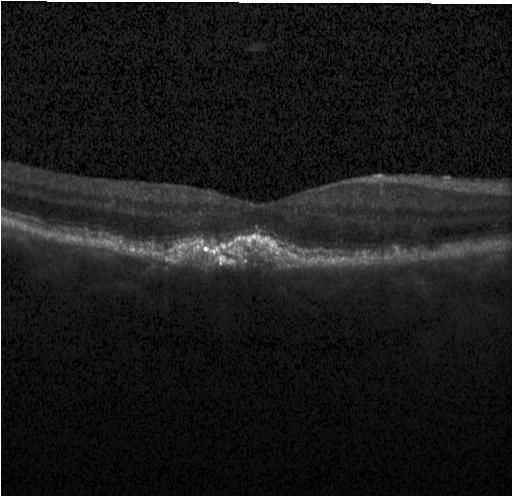 Heidelberg Spectralis OCT system · optical coherence tomography B-scan. The scan shows a choroidal neovascular membrane.